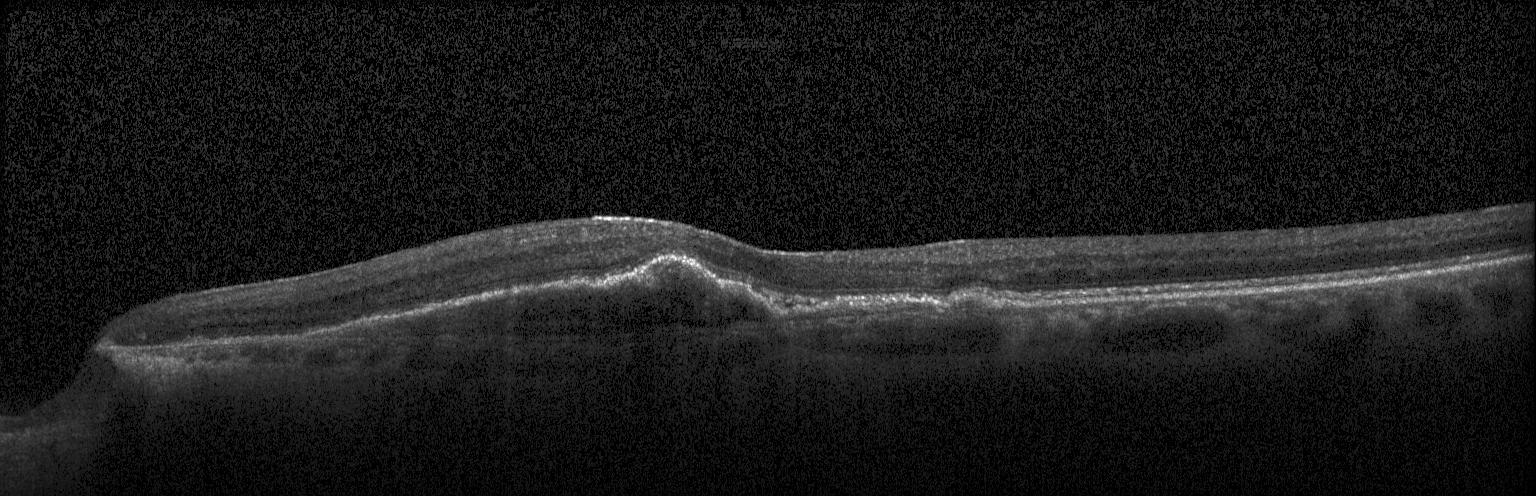
Heidelberg Spectralis. Optical coherence tomography B-scan. Finding: choroidal neovascularization.